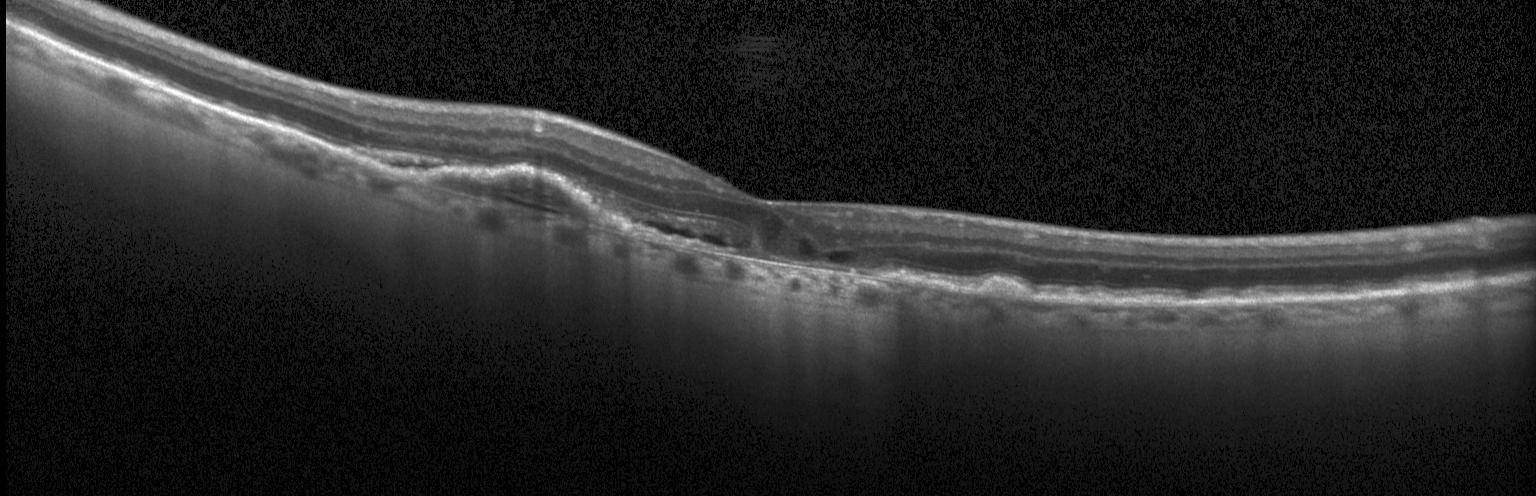 Retinal OCT B-scan, macular scan
Dx: a choroidal neovascular membrane.